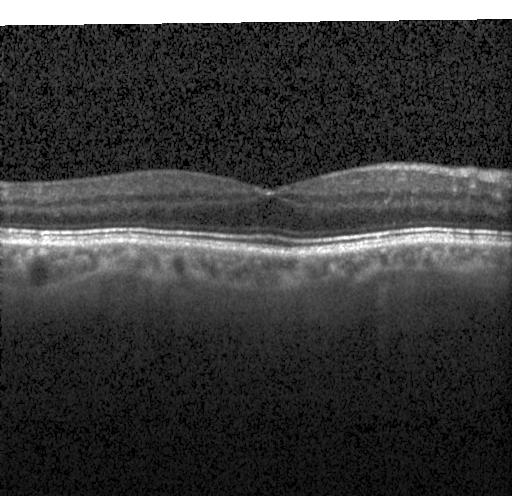 Instrument: Heidelberg Spectralis, horizontal scan through the fovea, OCT B-scan. Impression: neither CNV, DME, nor drusen.